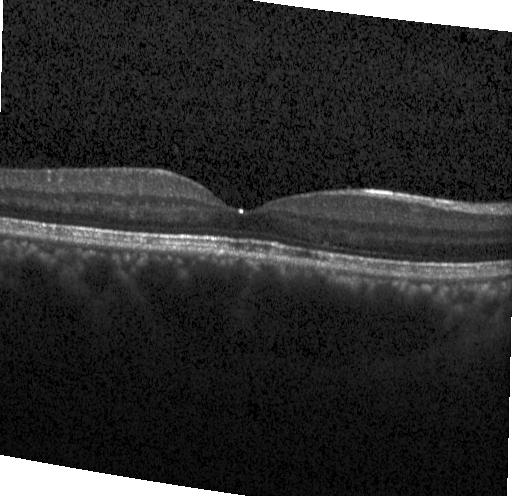 Macular OCT: no evidence of choroidal neovascularization, diabetic macular edema, or drusen.